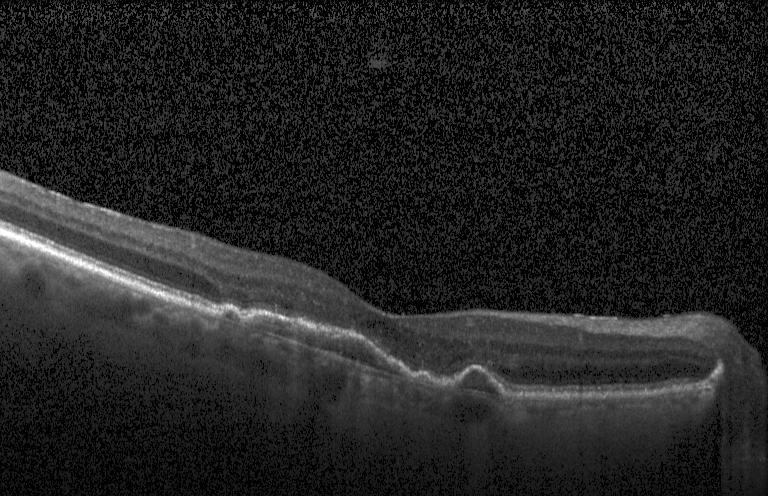
OCT B-scan. CNV.